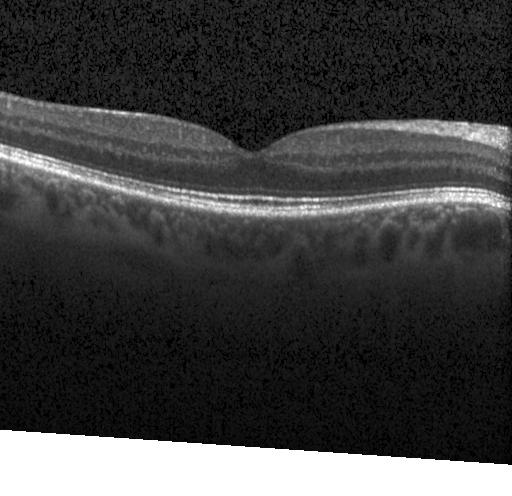

OCT line scan.
Diagnosis: neither CNV, DME, nor drusen.